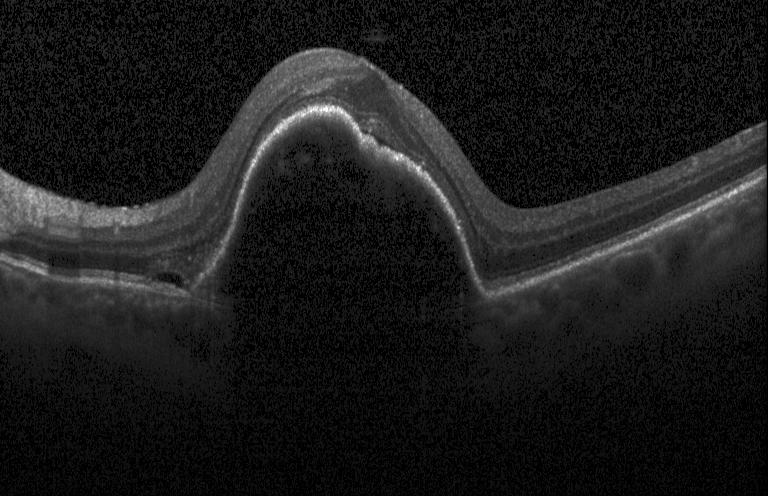

Finding: a choroidal neovascular membrane.